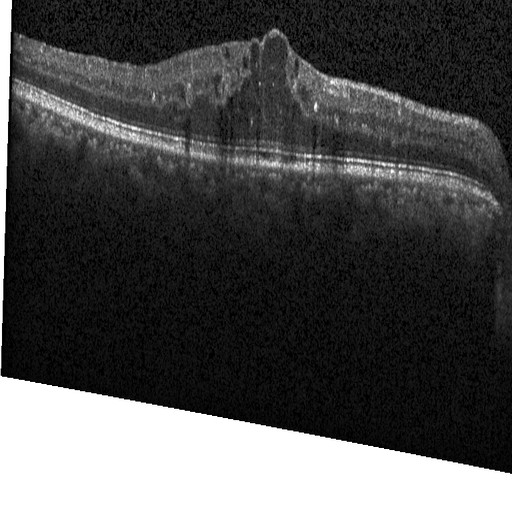 Spectral-domain optical coherence tomography; optical coherence tomography scan.
Macular OCT: diabetic macular edema.